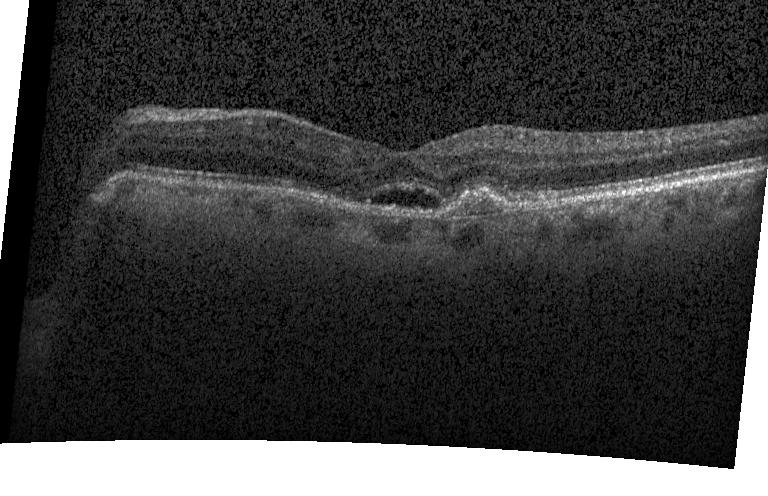
OCT line scan · spectral-domain optical coherence tomography · centered on the fovea.
Finding: a choroidal neovascular membrane.